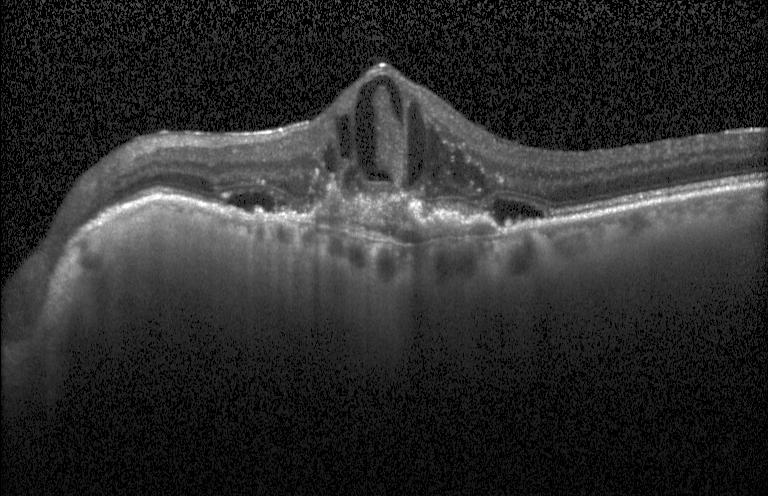

Heidelberg Spectralis · spectral-domain optical coherence tomography · OCT B-scan · fovea-centered — OCT finding: a choroidal neovascular membrane.